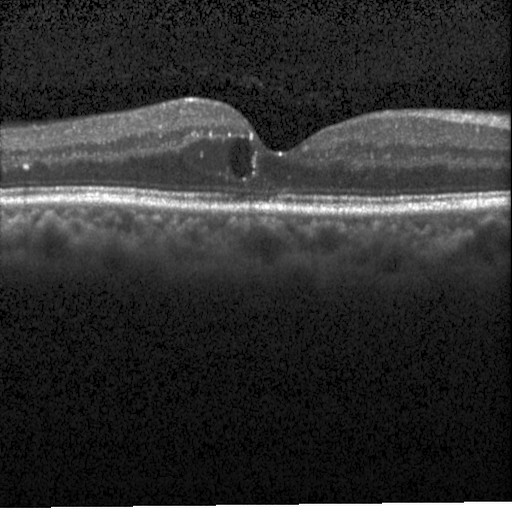

Optical coherence tomography B-scan, centered on the fovea. OCT finding: diabetic macular edema.